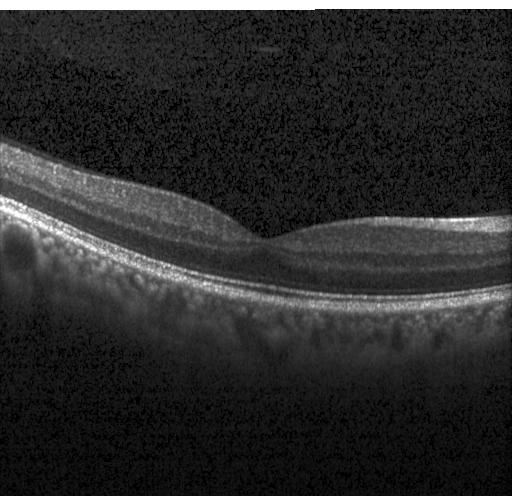

Spectral-domain OCT B-scan: no CNV, no DME, and no drusen.